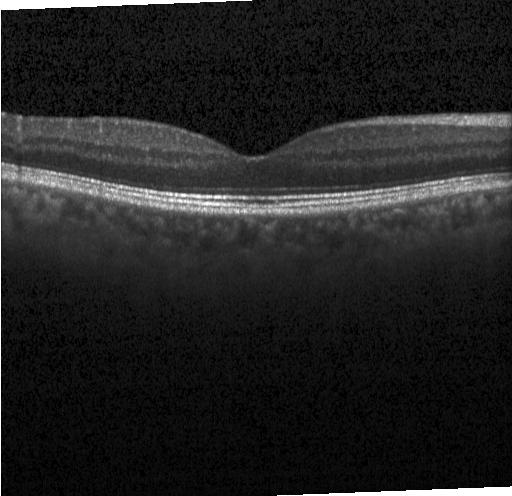
Spectral-domain OCT B-scan: neither choroidal neovascularization, diabetic macular edema, nor drusen.